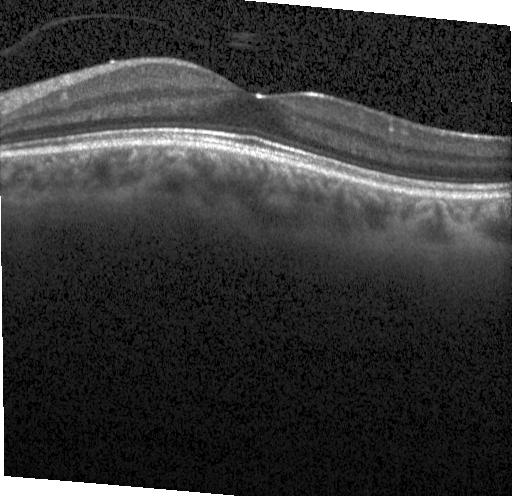
OCT scan showing no evidence of CNV, DME, or drusen.